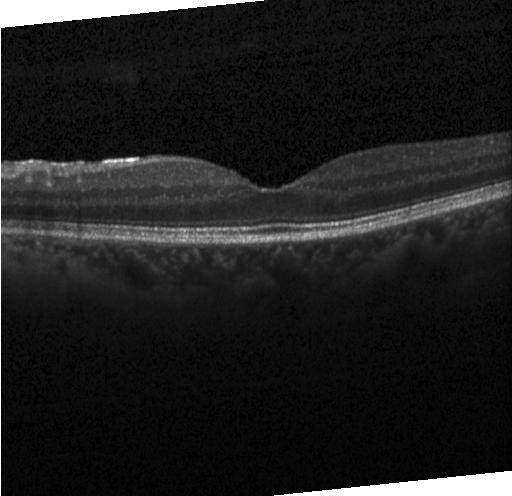 OCT finding: neither choroidal neovascularization, diabetic macular edema, nor drusen.